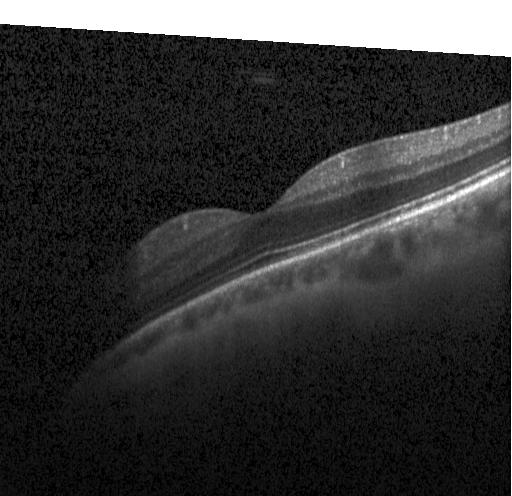
Finding: no CNV, no DME, and no drusen.